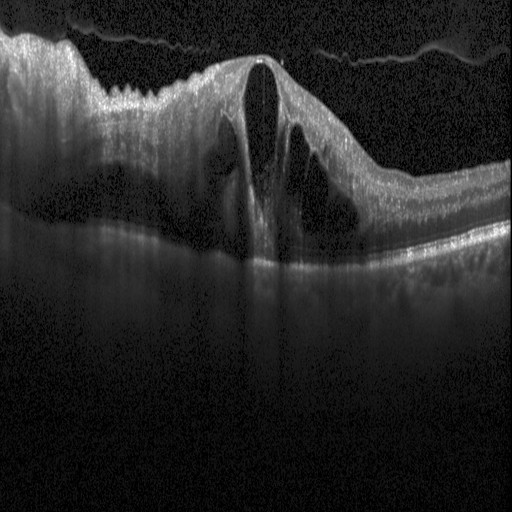
Retinal OCT cross-section.
Impression: diabetic macular edema (DME).